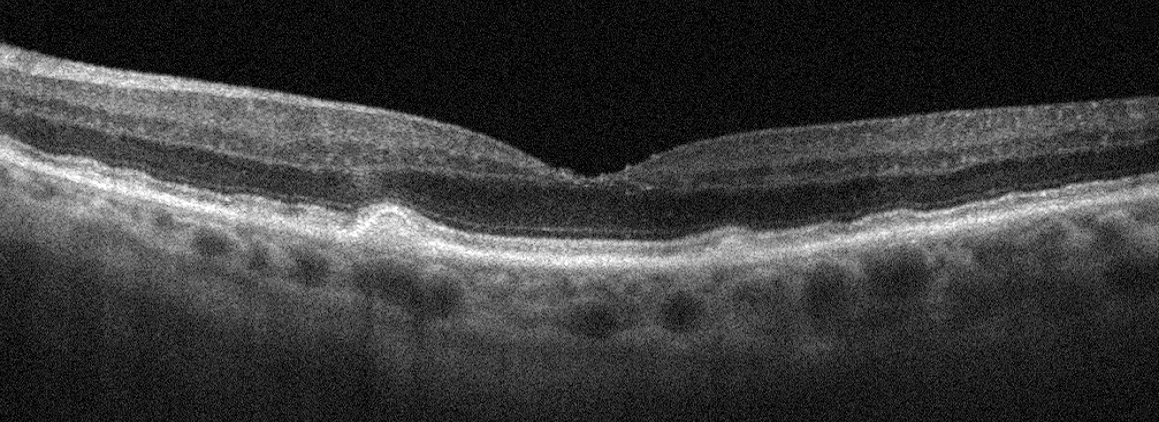 Through the macula · instrument: Optovue Avanti RTVue XR · oculus sinister · optical coherence tomography B-scan — Age-related macular degeneration (AMD).